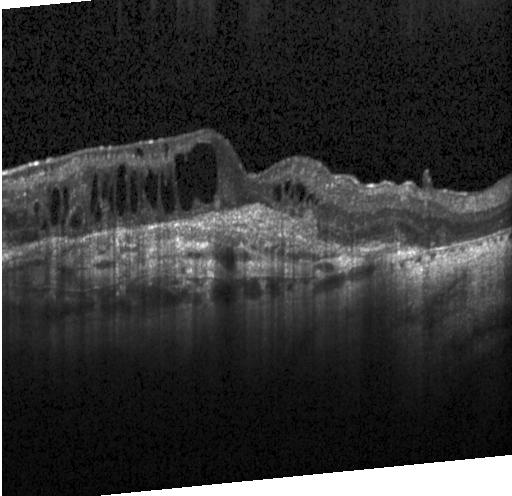

Centered on the fovea; retinal OCT B-scan
Macular OCT: a choroidal neovascular membrane.